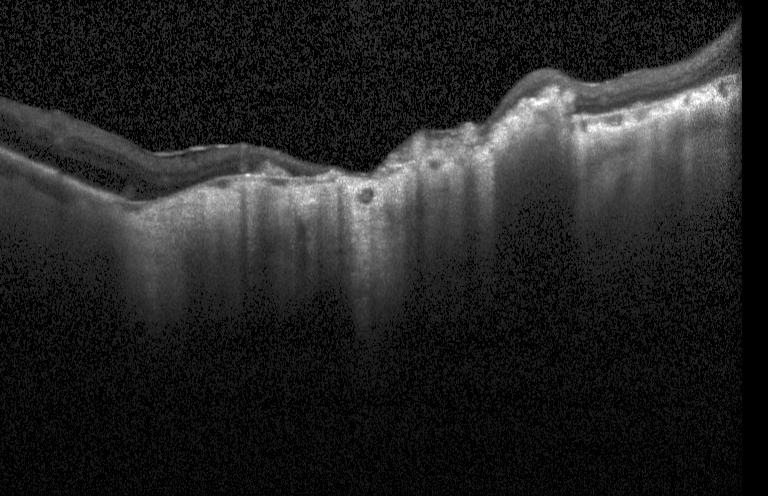 Retinal OCT B-scan, acquired on a Heidelberg Spectralis. Dx: a choroidal neovascular membrane.